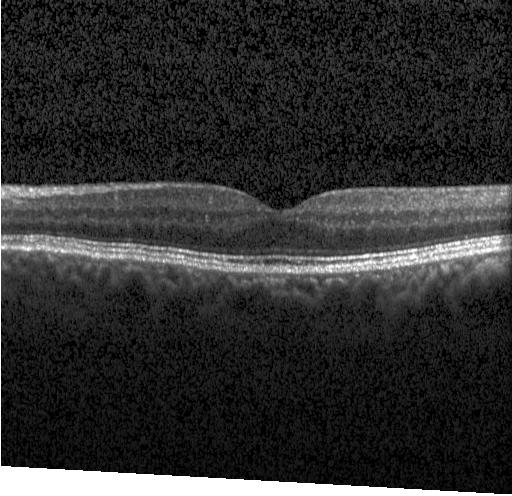

Optical coherence tomography scan · spectral-domain OCT. Impression: no evidence of choroidal neovascularization, diabetic macular edema, or drusen.